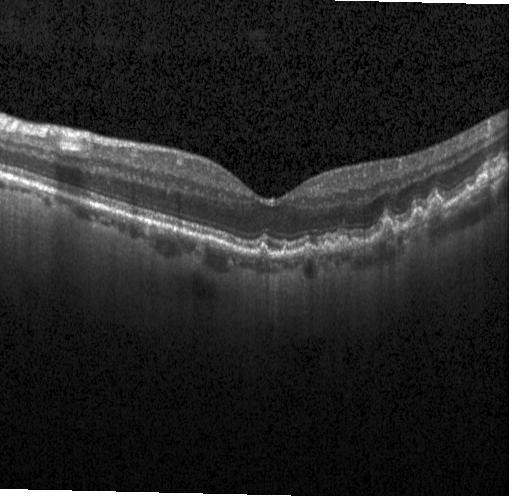
Impression: sub-RPE drusenoid deposits.